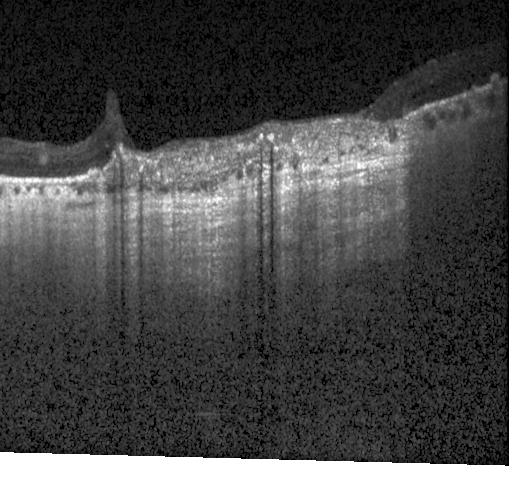 Horizontal scan through the fovea. Retinal OCT cross-section
Diagnosis: choroidal neovascularization (CNV).